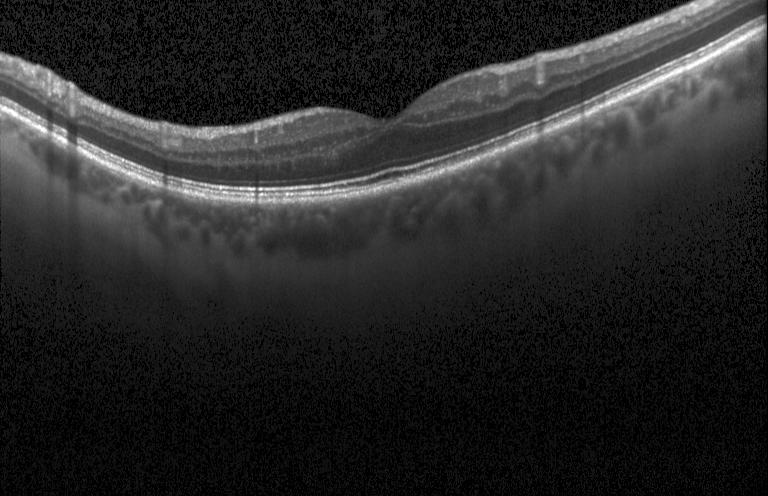

Dx: no evidence of CNV, DME, or drusen.